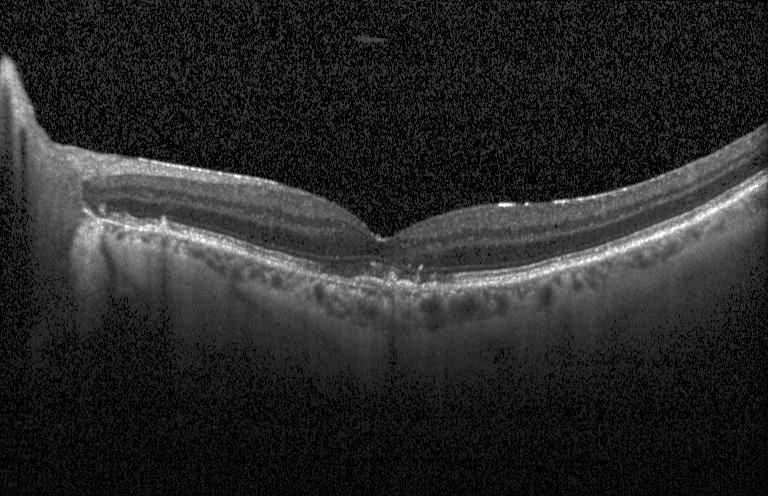 Optical coherence tomography B-scan; fovea-centered. Finding: a choroidal neovascular membrane.